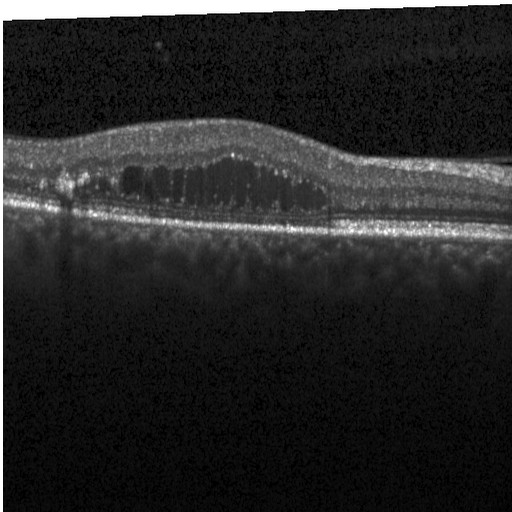
This B-scan demonstrates diabetic macular edema.